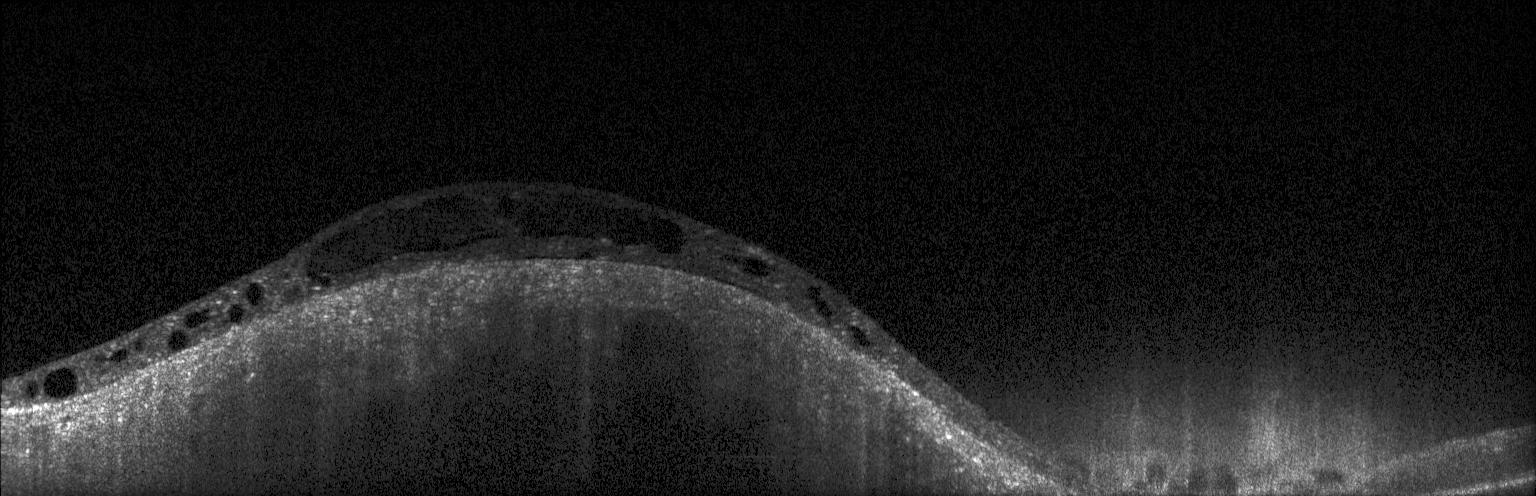
Macular OCT: diabetic macular edema (DME).